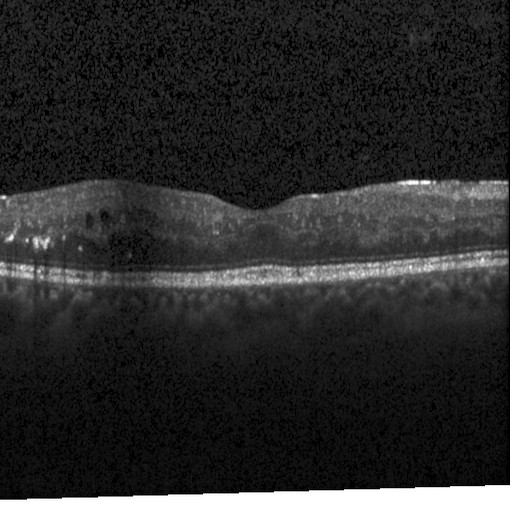
OCT finding: diabetic macular edema (DME).